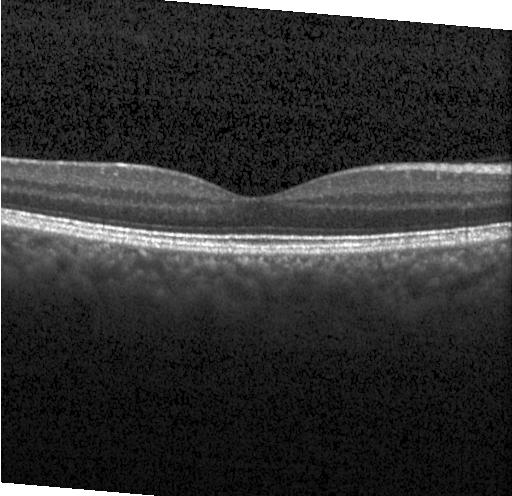

Instrument: Heidelberg Spectralis. Optical coherence tomography scan — Diagnosis: no choroidal neovascularization, no diabetic macular edema, and no drusen.